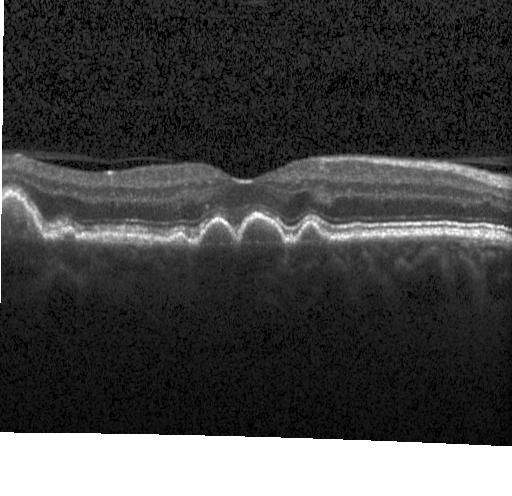 Optical coherence tomography scan, acquired on a Heidelberg Spectralis.
Finding: sub-RPE drusenoid deposits.